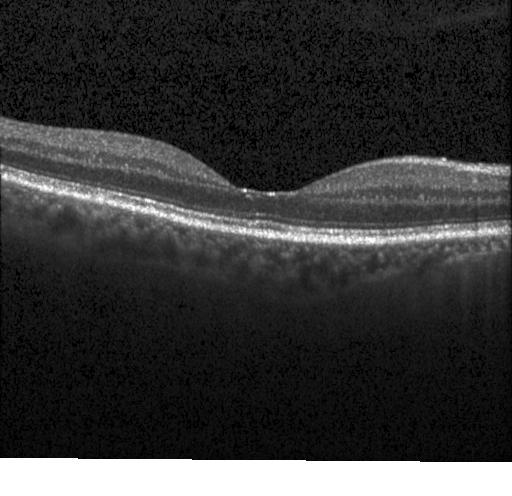 Through the macula; spectral-domain OCT; retinal OCT cross-section; Heidelberg Spectralis OCT system — The scan shows neither choroidal neovascularization, diabetic macular edema, nor drusen.